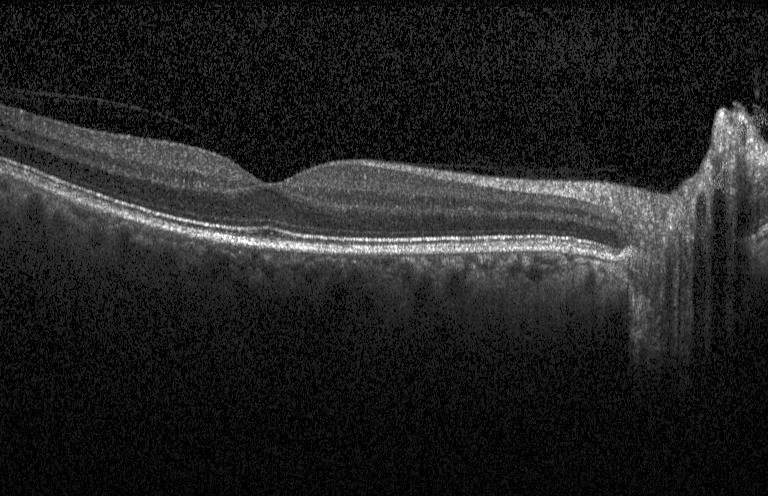
Spectral-domain OCT B-scan: no choroidal neovascularization, diabetic macular edema, or drusen.